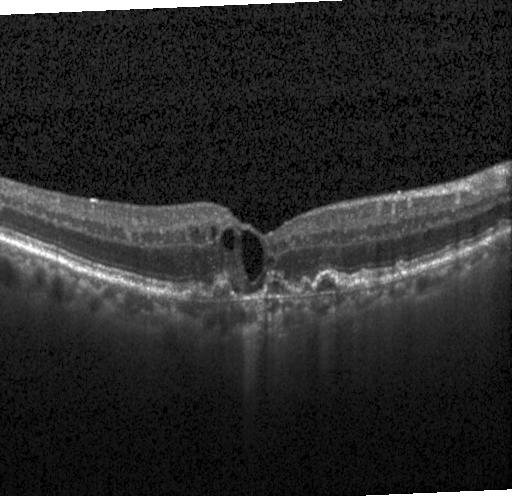

Finding: choroidal neovascularization.